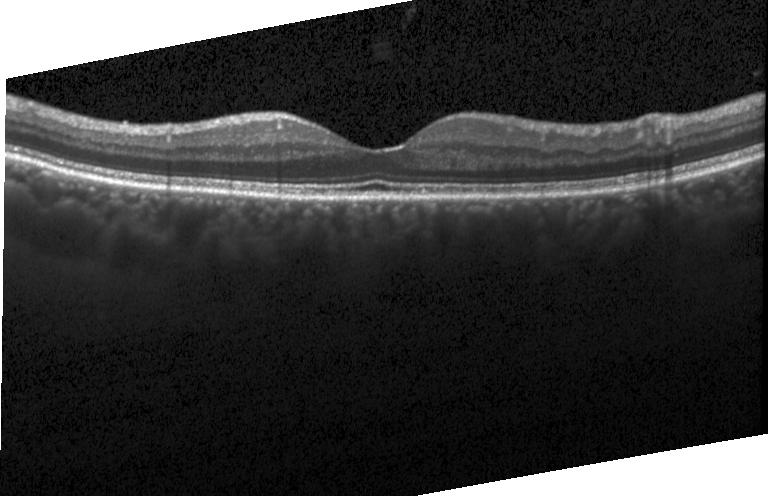

Impression: no choroidal neovascularization, no diabetic macular edema, and no drusen.